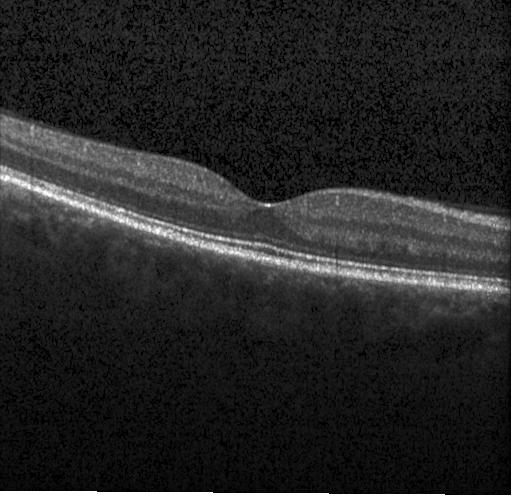
The scan shows no choroidal neovascularization, diabetic macular edema, or drusen.